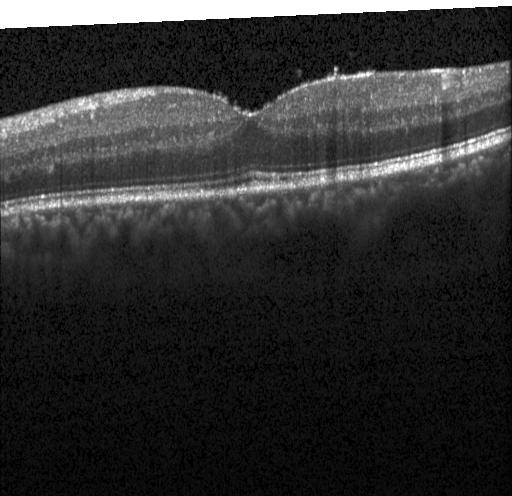

OCT line scan — The scan shows no choroidal neovascularization, no diabetic macular edema, and no drusen.